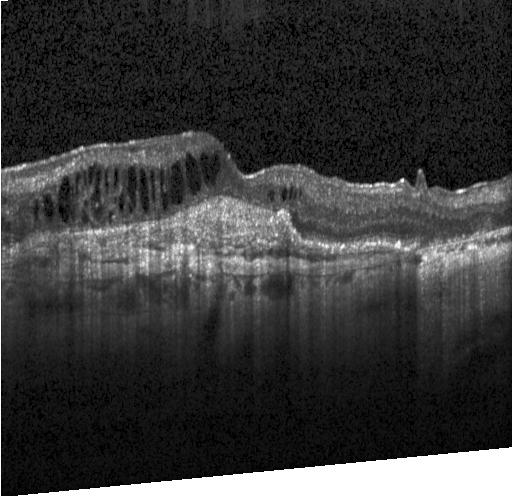
Acquired on a Heidelberg Spectralis · optical coherence tomography B-scan · spectral-domain optical coherence tomography · macular scan.
The scan shows choroidal neovascularization.